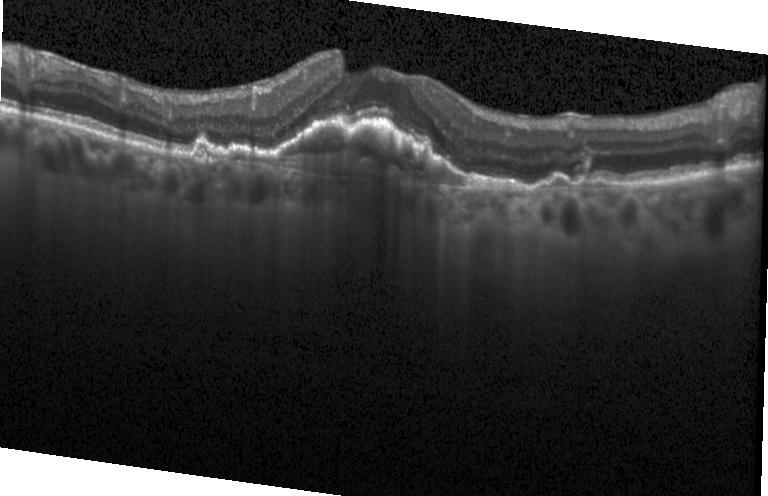

Retinal OCT cross-section showing a choroidal neovascular membrane.